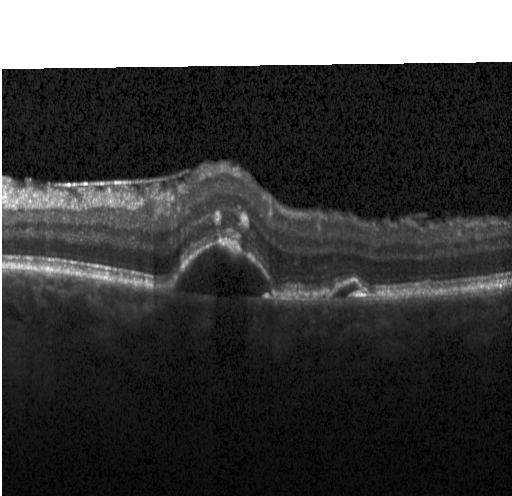 Dx: choroidal neovascularization (CNV).